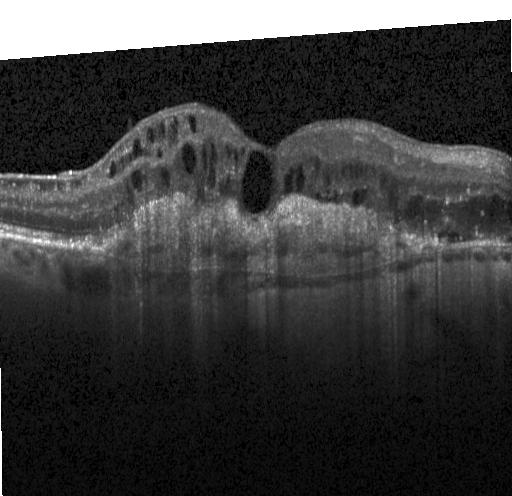
Diagnosis: a choroidal neovascular membrane.